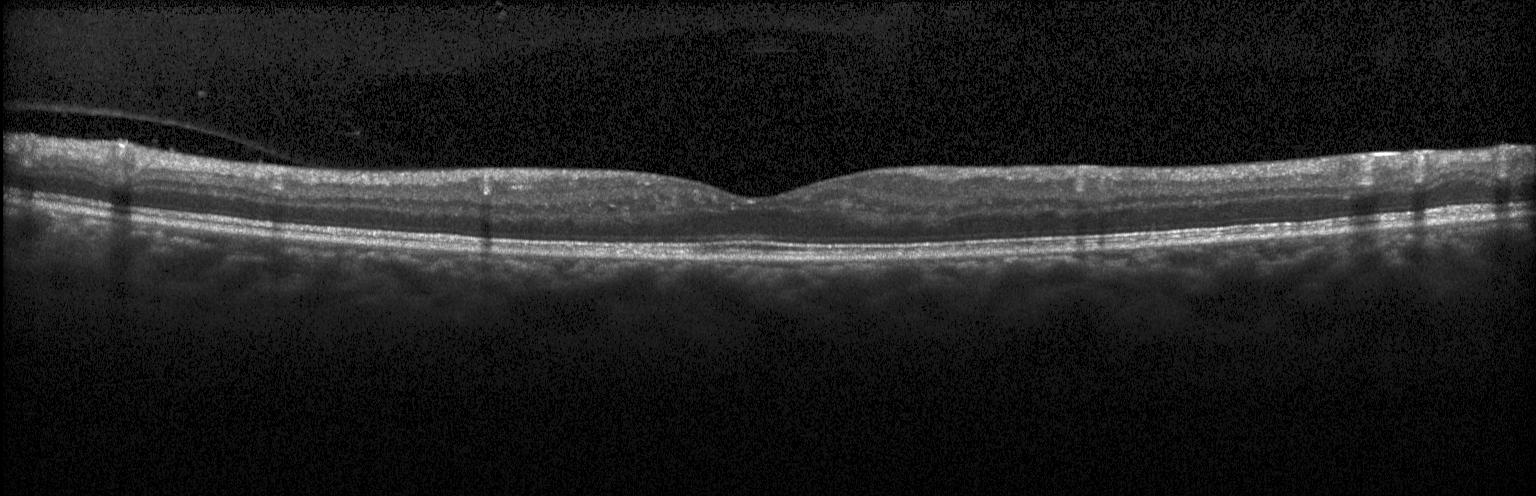
Instrument: Heidelberg Spectralis · spectral-domain OCT · through the macula · optical coherence tomography B-scan
The scan shows no CNV, DME, or drusen.